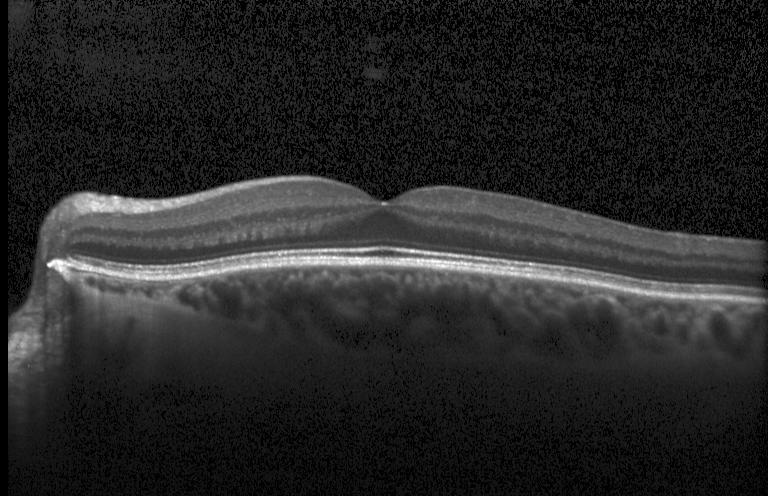
Optical coherence tomography scan
Impression: no evidence of choroidal neovascularization, diabetic macular edema, or drusen.